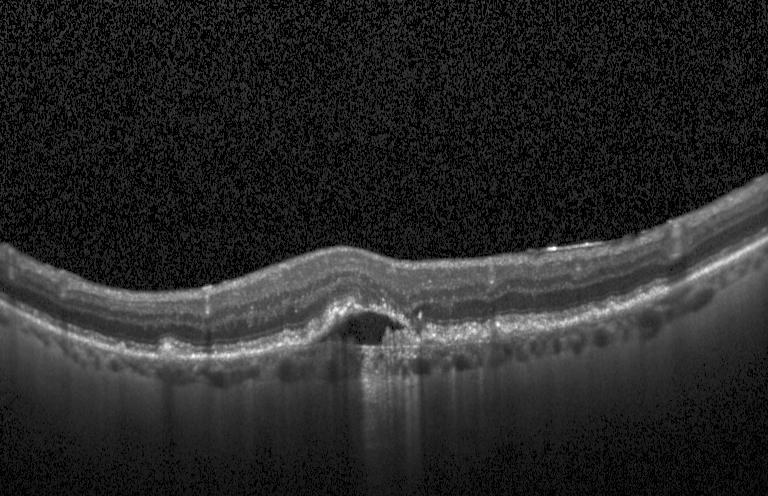
Through the macula · optical coherence tomography scan · Heidelberg Spectralis OCT system. Diagnosis: choroidal neovascularization.